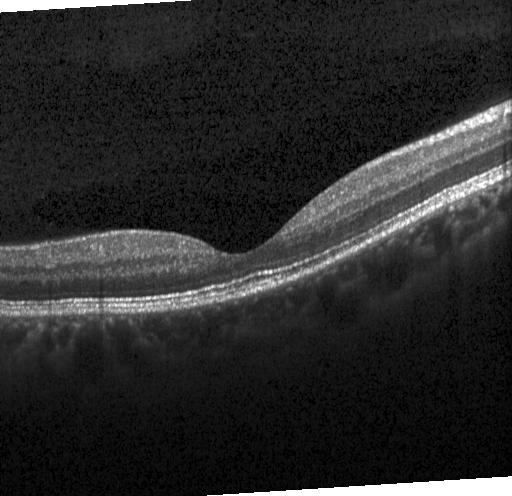 OCT scan showing no choroidal neovascularization, diabetic macular edema, or drusen.